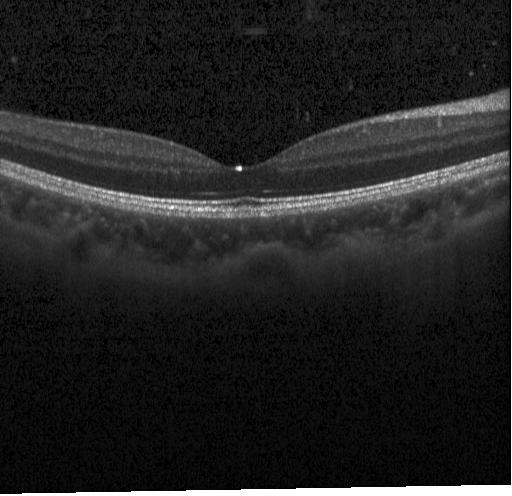 SD-OCT; fovea-centered; Heidelberg Spectralis; retinal OCT B-scan — Finding: no CNV, DME, or drusen.